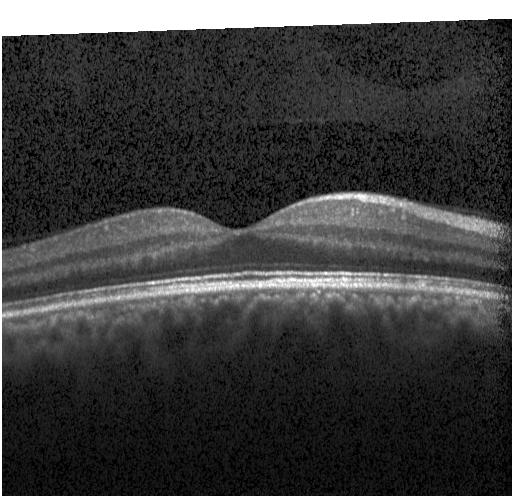
Diagnosis: no evidence of choroidal neovascularization, diabetic macular edema, or drusen.